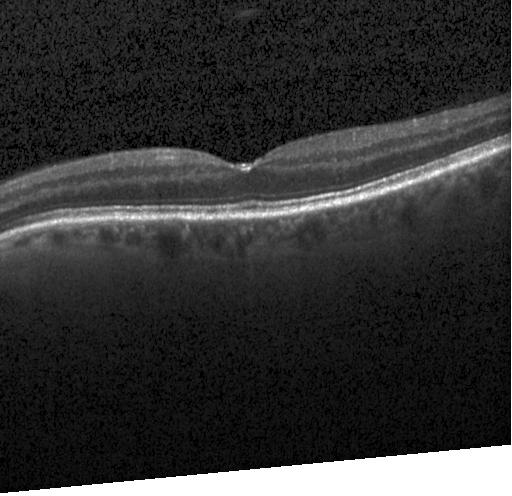
Heidelberg Spectralis. Optical coherence tomography B-scan.
Finding: no evidence of choroidal neovascularization, diabetic macular edema, or drusen.